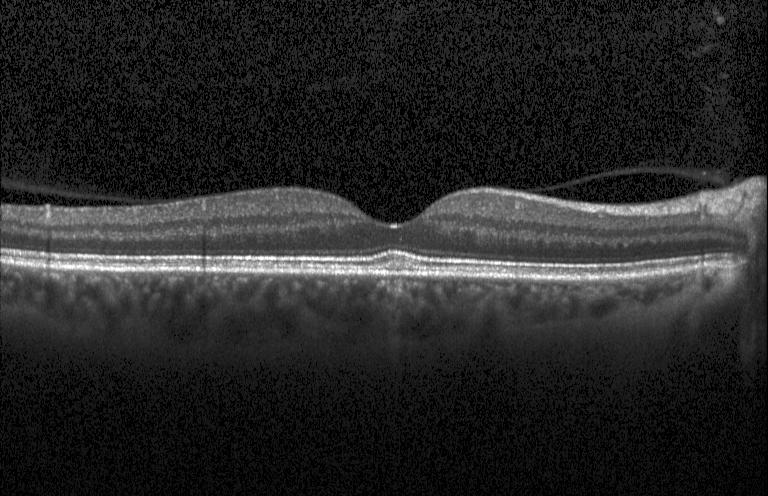

OCT scan showing neither choroidal neovascularization, diabetic macular edema, nor drusen.